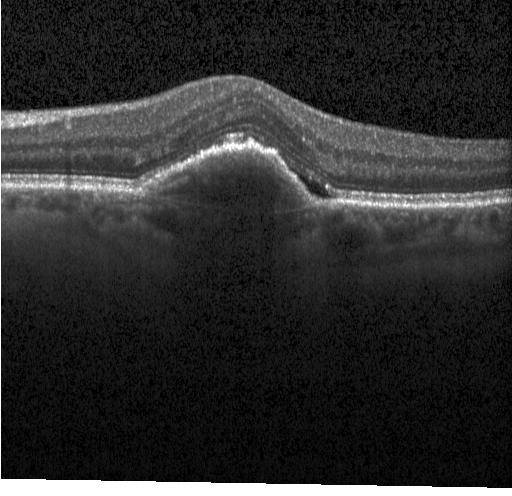 Retinal OCT cross-section — Macular OCT: choroidal neovascularization.